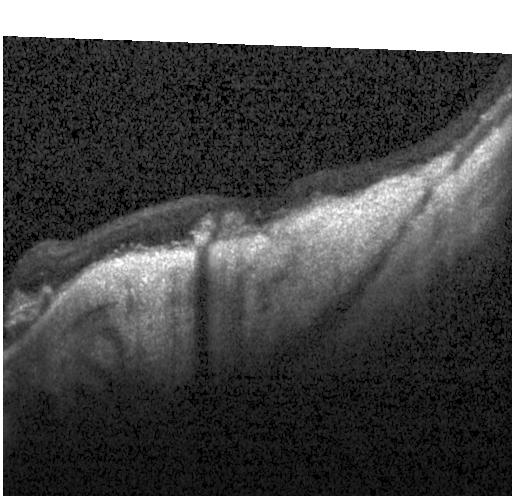

Finding: a choroidal neovascular membrane.